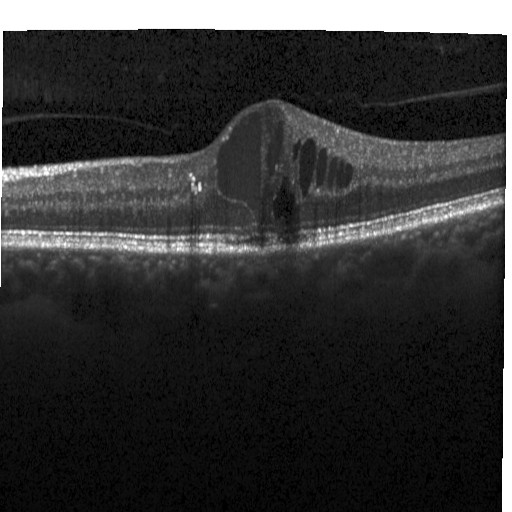
Macular OCT: diabetic macular edema (DME).